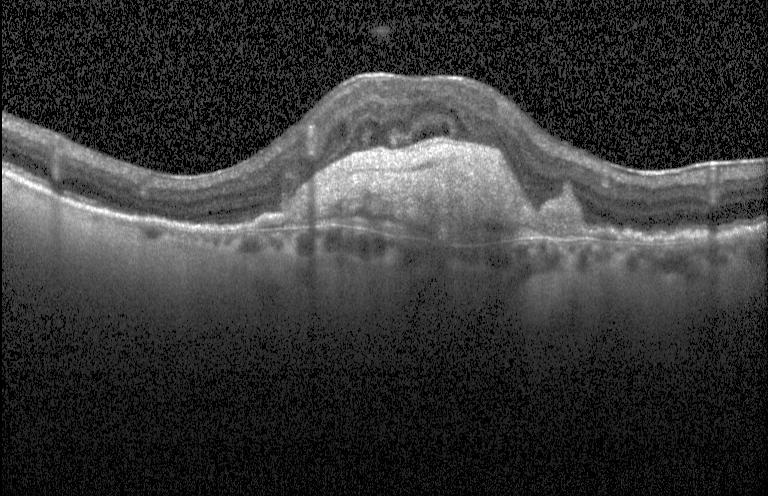
OCT scan showing a choroidal neovascular membrane.